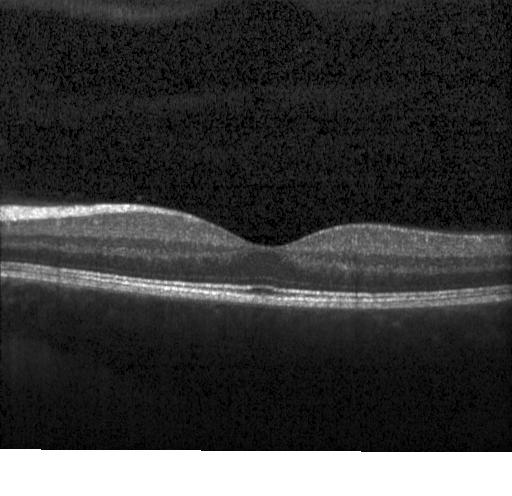
Optical coherence tomography scan.
Finding: no choroidal neovascularization, no diabetic macular edema, and no drusen.